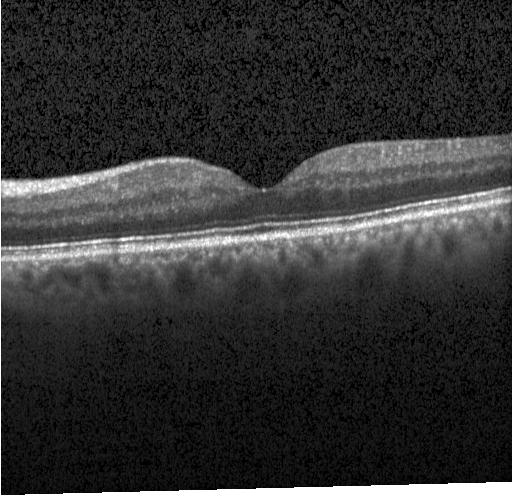

Assessment: no evidence of choroidal neovascularization, diabetic macular edema, or drusen.